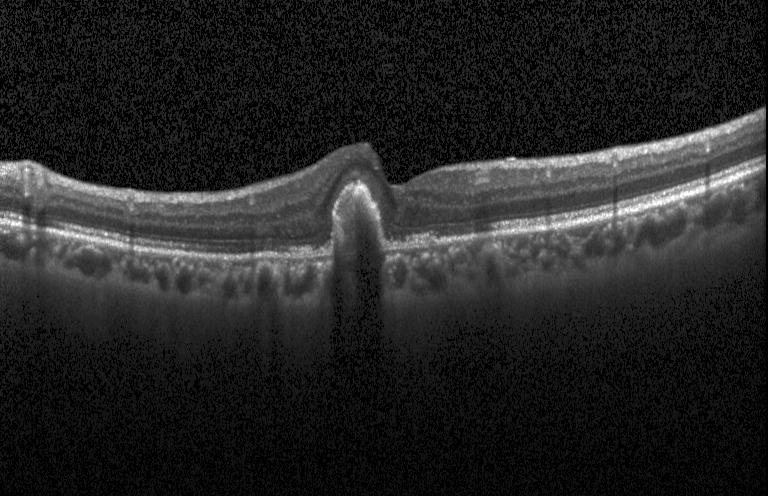 Diagnosis: a choroidal neovascular membrane.